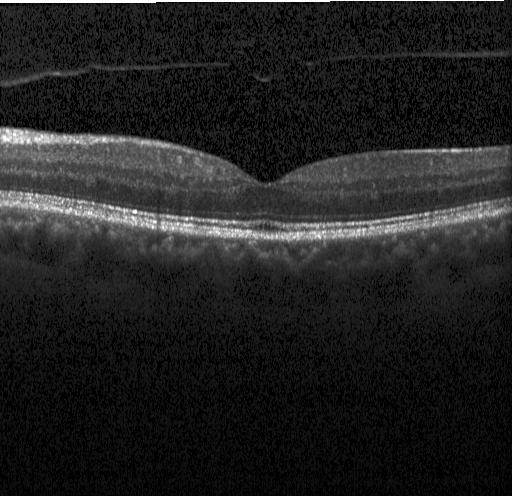
Impression: no choroidal neovascularization, no diabetic macular edema, and no drusen.